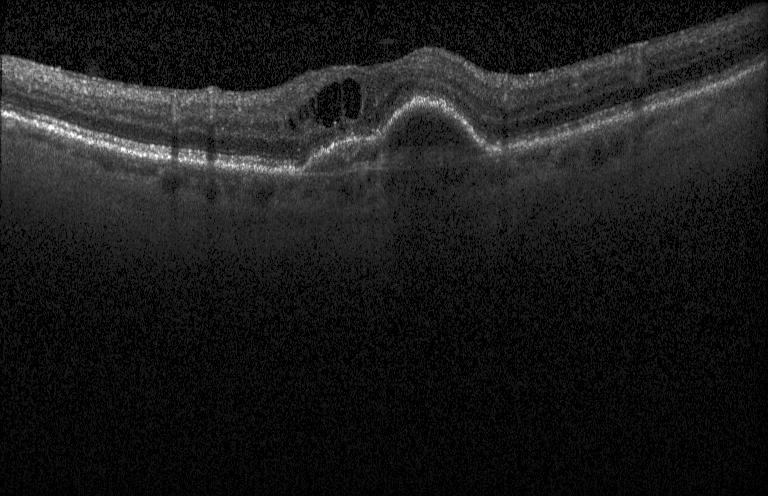 Instrument: Heidelberg Spectralis; OCT line scan; horizontal scan through the fovea; SD-OCT — Impression: CNV.